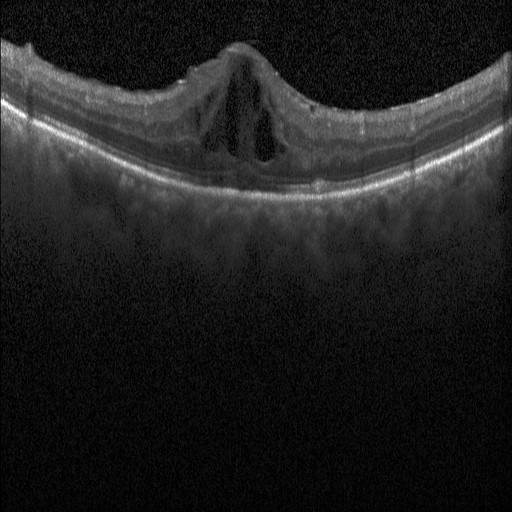
OCT B-scan showing diabetic macular edema (DME).